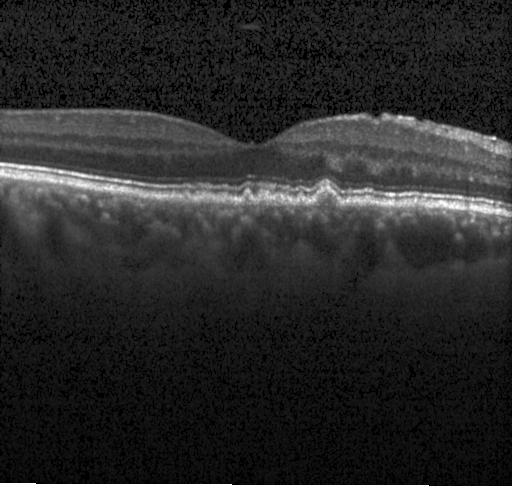

Centered on the fovea. SD-OCT. Acquired on a Heidelberg Spectralis. OCT line scan — Assessment: drusen.